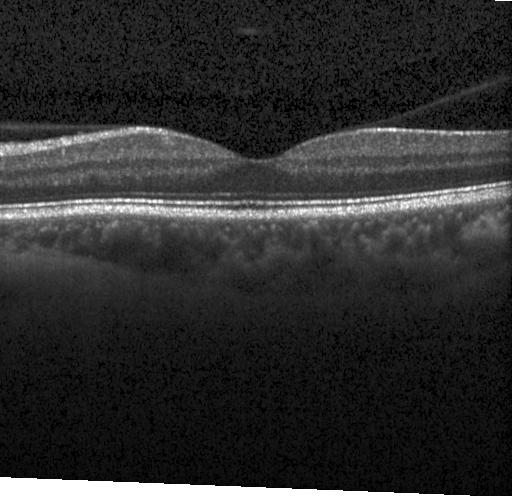 Optical coherence tomography scan; fovea-centered — OCT finding: no CNV, DME, or drusen.